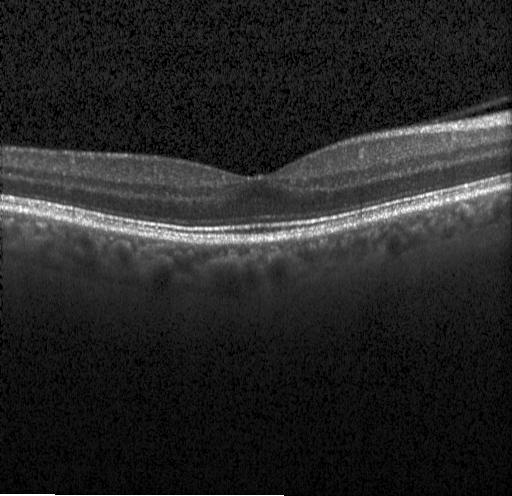

Optical coherence tomography scan, instrument: Heidelberg Spectralis
Diagnosis: no choroidal neovascularization, diabetic macular edema, or drusen.